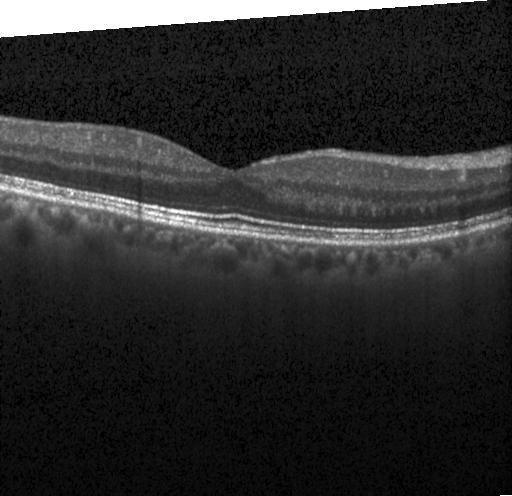

Retinal OCT cross-section
Impression: no choroidal neovascularization, no diabetic macular edema, and no drusen.